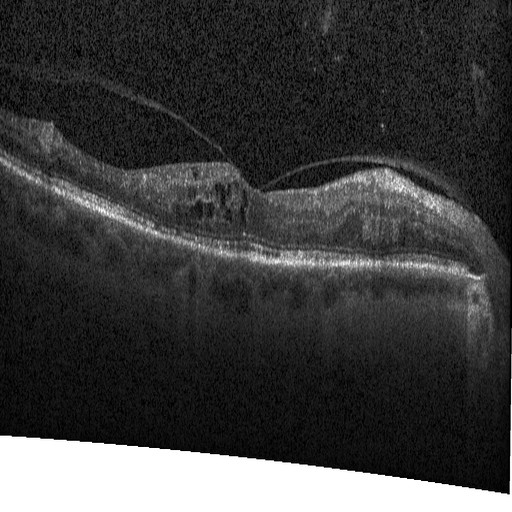 Impression: DME.